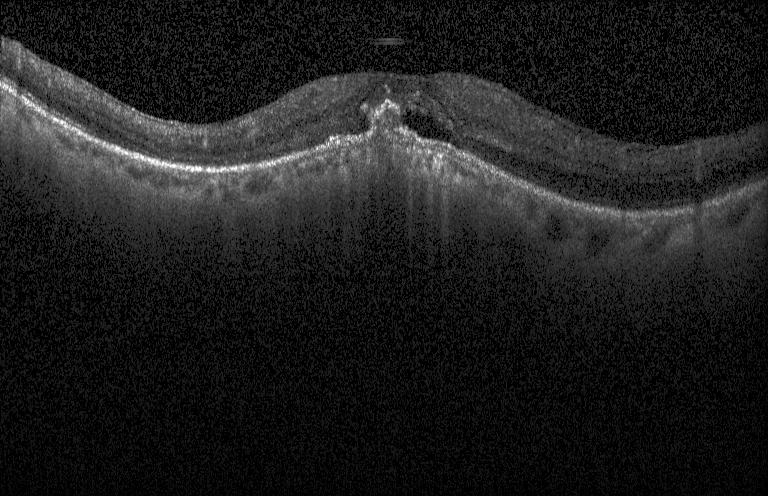 Macular scan. Optical coherence tomography scan.
A choroidal neovascular membrane.